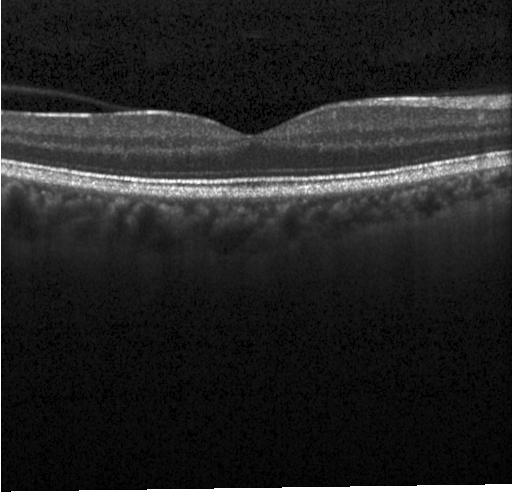 Retinal OCT cross-section. Centered on the fovea. Acquired on a Heidelberg Spectralis. SD-OCT.
Diagnosis: no choroidal neovascularization, diabetic macular edema, or drusen.